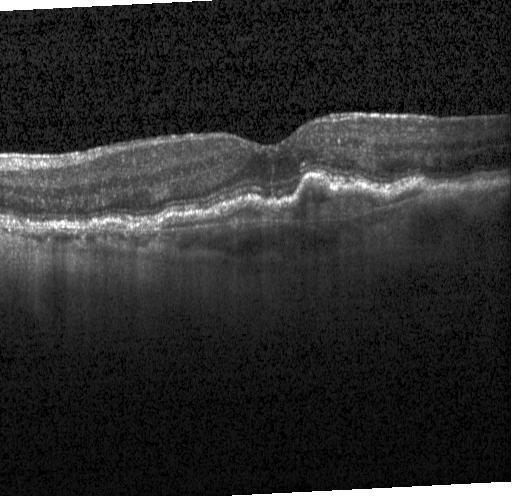
Fovea-centered; retinal OCT B-scan — OCT finding: choroidal neovascularization (CNV).